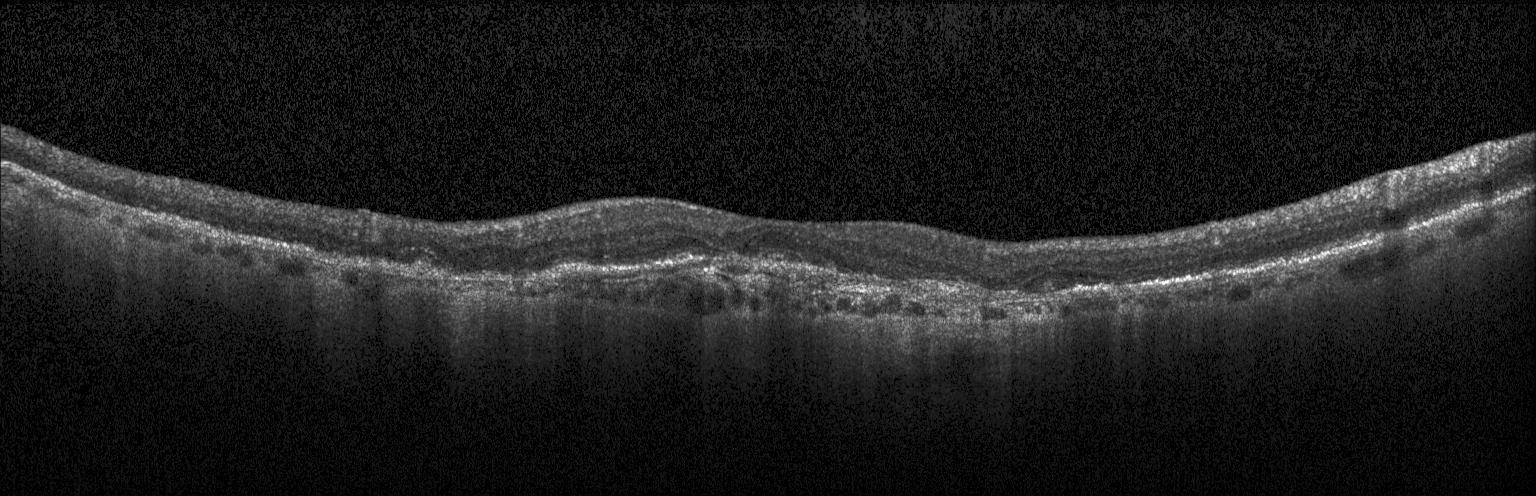
Optical coherence tomography scan — Diagnosis: choroidal neovascularization.